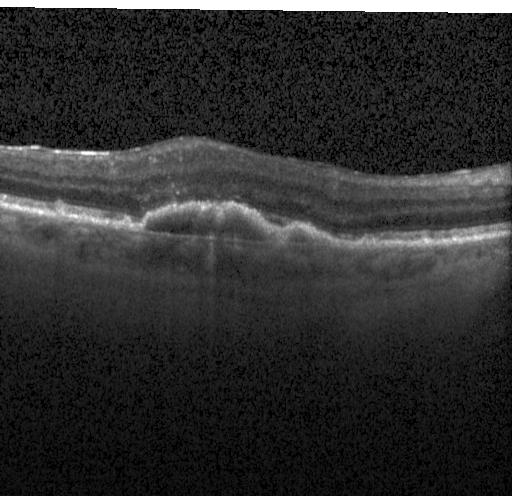

Diagnosis: CNV.